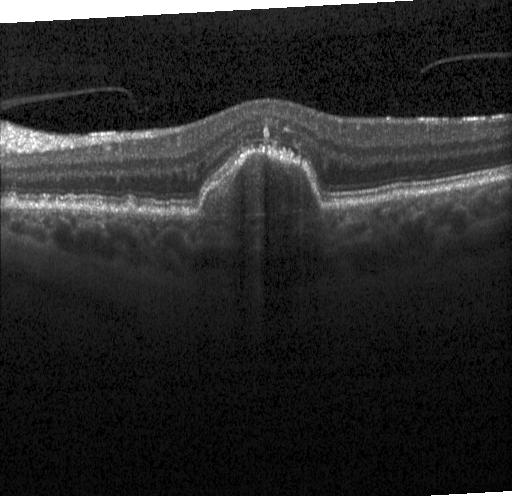
Diagnosis: a choroidal neovascular membrane.